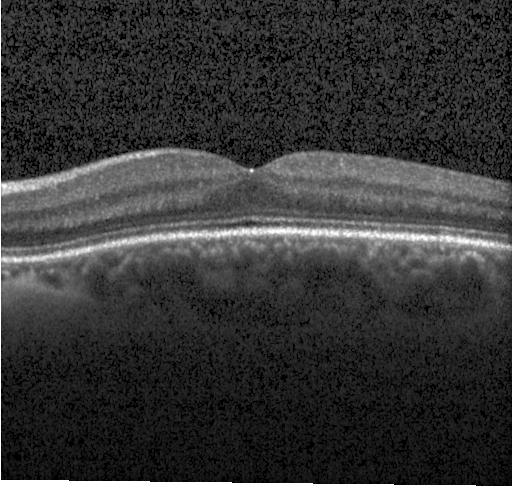

Retinal OCT cross-section, spectral-domain OCT. Finding: no CNV, no DME, and no drusen.